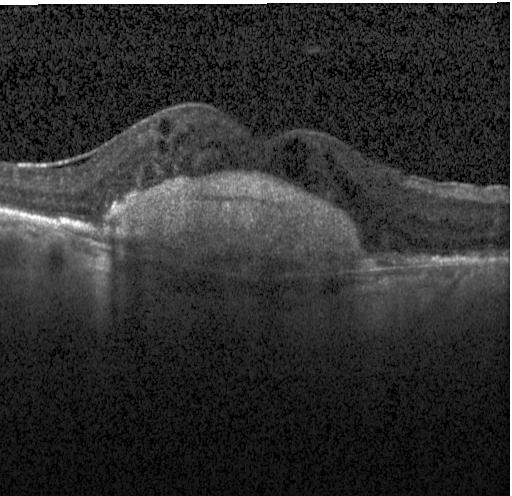

OCT line scan.
The scan shows a choroidal neovascular membrane.